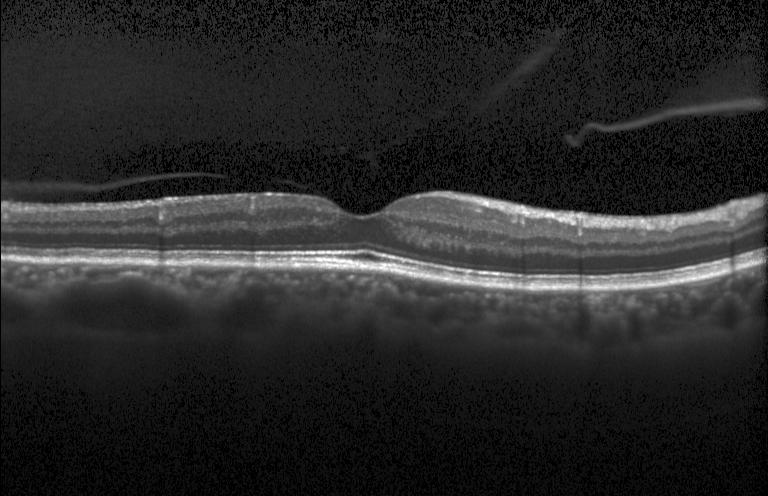
Spectral-domain OCT; retinal OCT cross-section.
Diagnosis: no choroidal neovascularization, no diabetic macular edema, and no drusen.